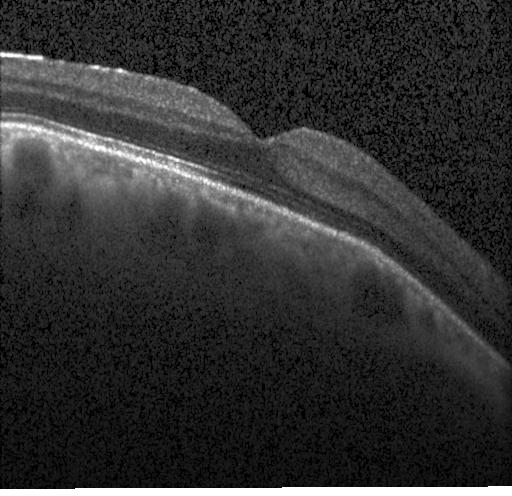
Assessment: no CNV, DME, or drusen.